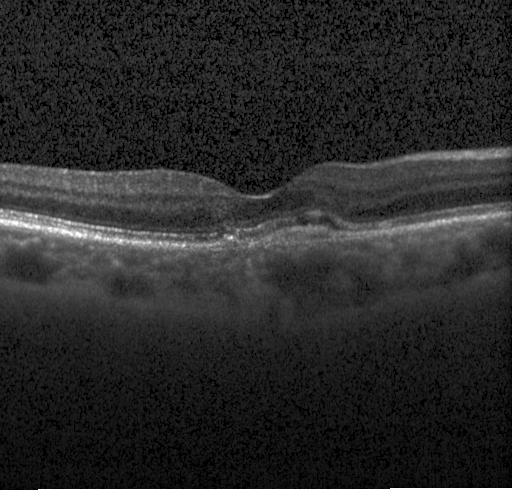
Assessment: choroidal neovascularization (CNV).